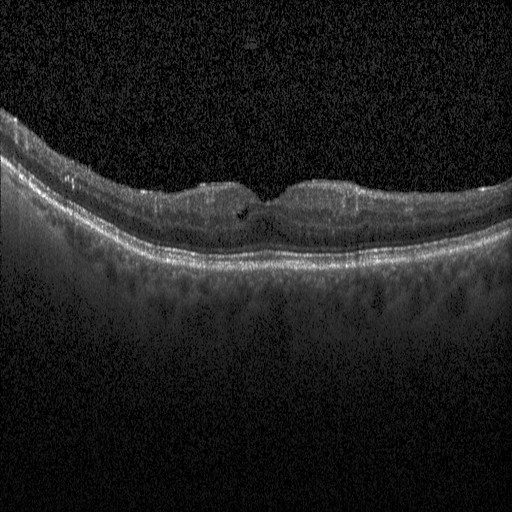 Spectral-domain optical coherence tomography · retinal OCT cross-section.
The scan shows diabetic macular edema.